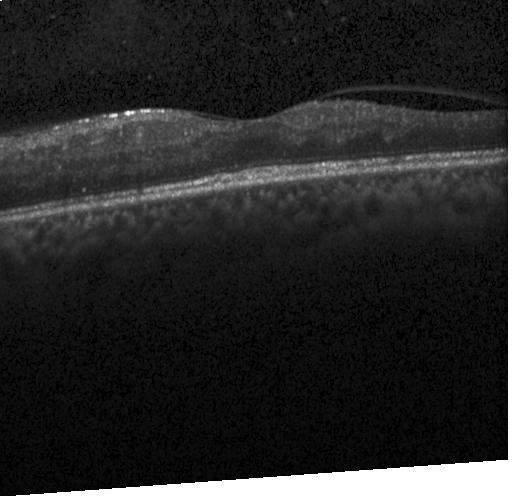 Retinal OCT B-scan · Heidelberg Spectralis OCT system · centered on the fovea.
This B-scan demonstrates diabetic macular edema.